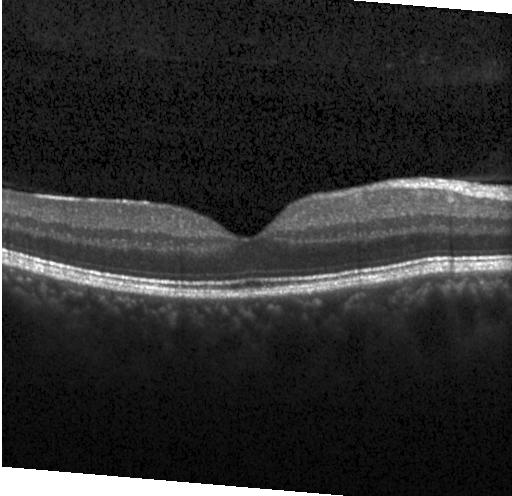 Macular OCT demonstrating no CNV, DME, or drusen.